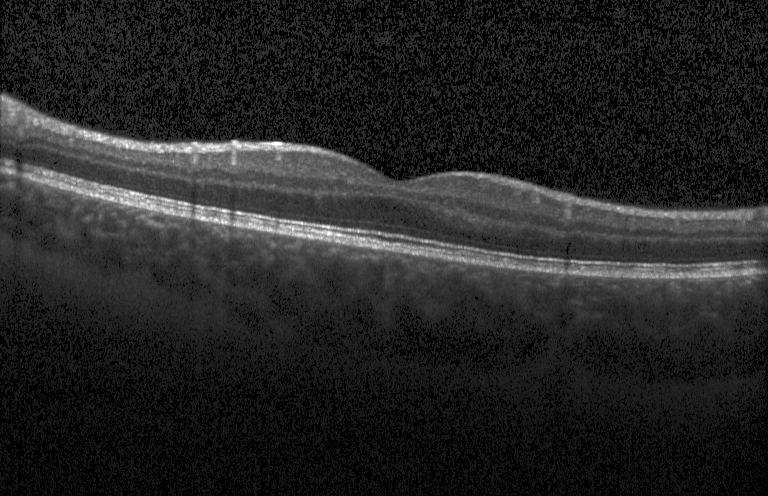
Dx: neither CNV, DME, nor drusen.